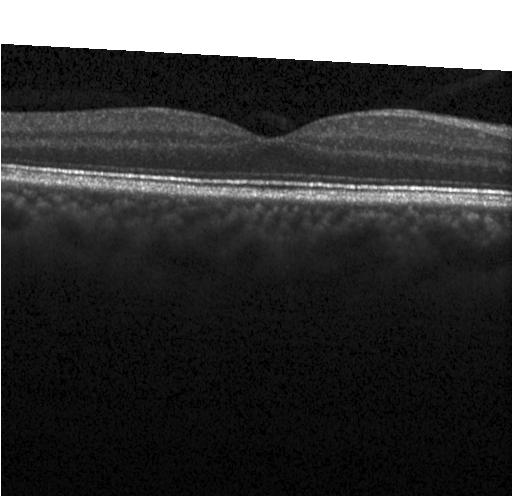 Spectral-domain OCT; OCT line scan — The scan shows neither choroidal neovascularization, diabetic macular edema, nor drusen.